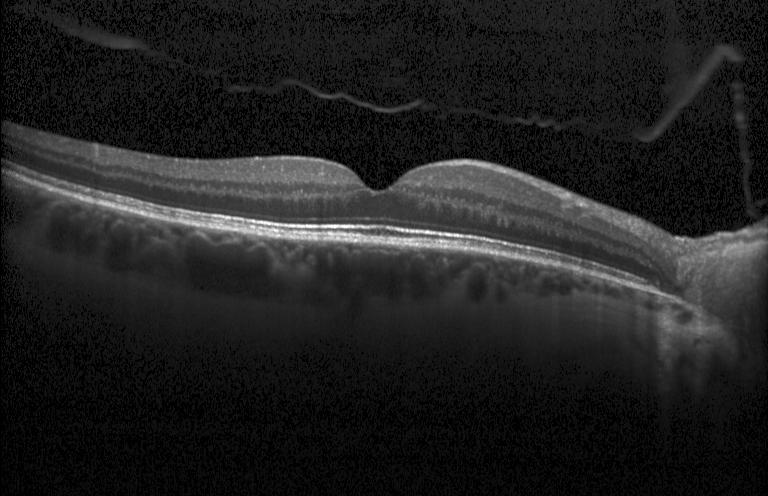

Optical coherence tomography scan.
The scan shows neither CNV, DME, nor drusen.